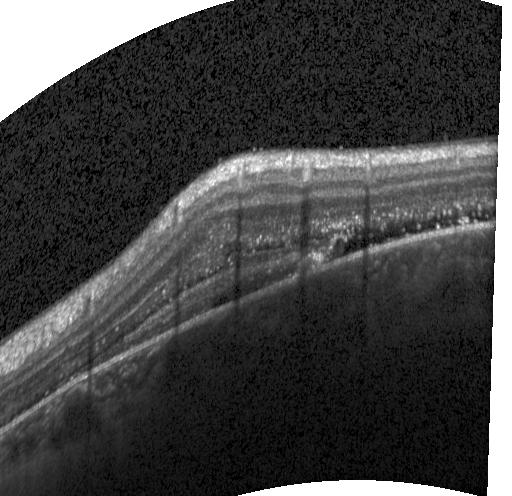

OCT line scan · spectral-domain optical coherence tomography · instrument: Heidelberg Spectralis — Impression: CNV.